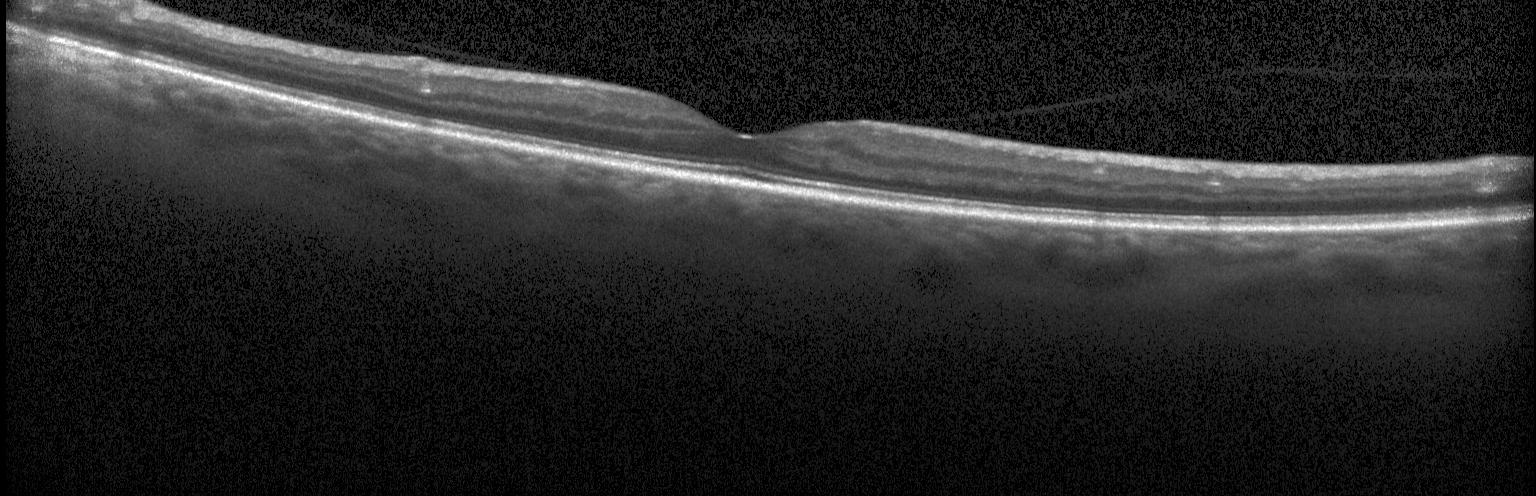
Spectral-domain OCT, acquired on a Heidelberg Spectralis, retinal OCT B-scan, macular scan. The scan shows no choroidal neovascularization, diabetic macular edema, or drusen.